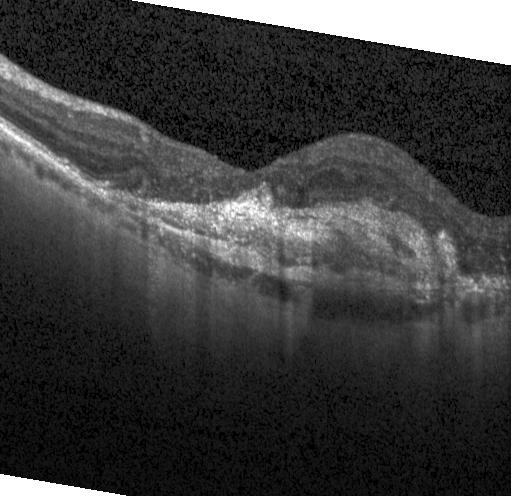 Optical coherence tomography B-scan.
Finding: a choroidal neovascular membrane.